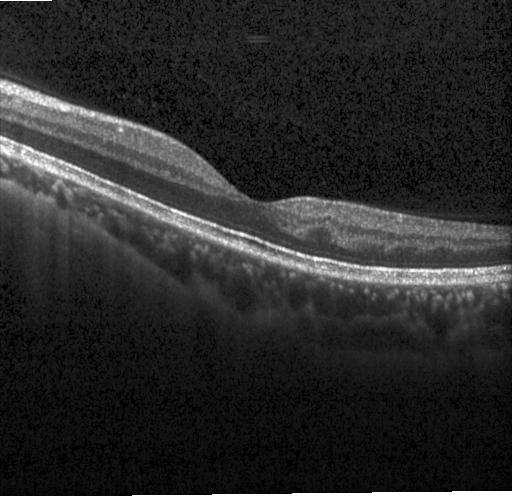 Dx: no choroidal neovascularization, no diabetic macular edema, and no drusen.